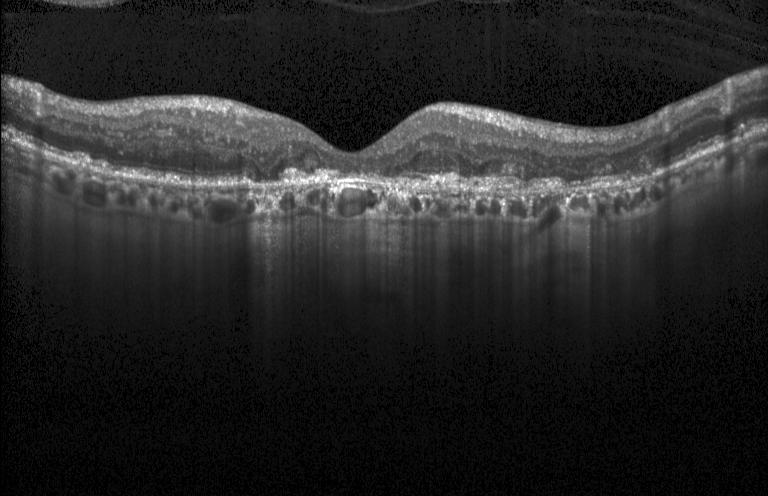 Dx: choroidal neovascularization.